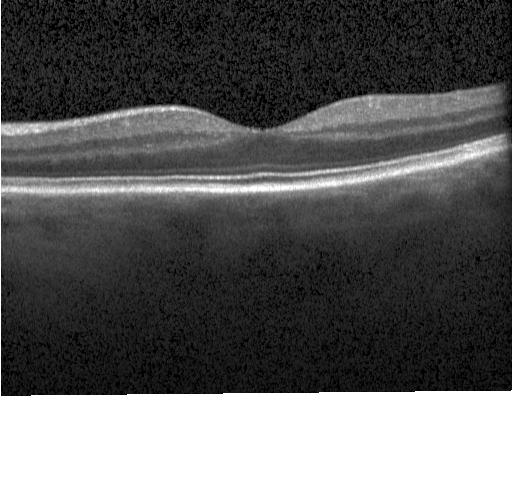 Fovea-centered · OCT B-scan · SD-OCT
Finding: no evidence of choroidal neovascularization, diabetic macular edema, or drusen.